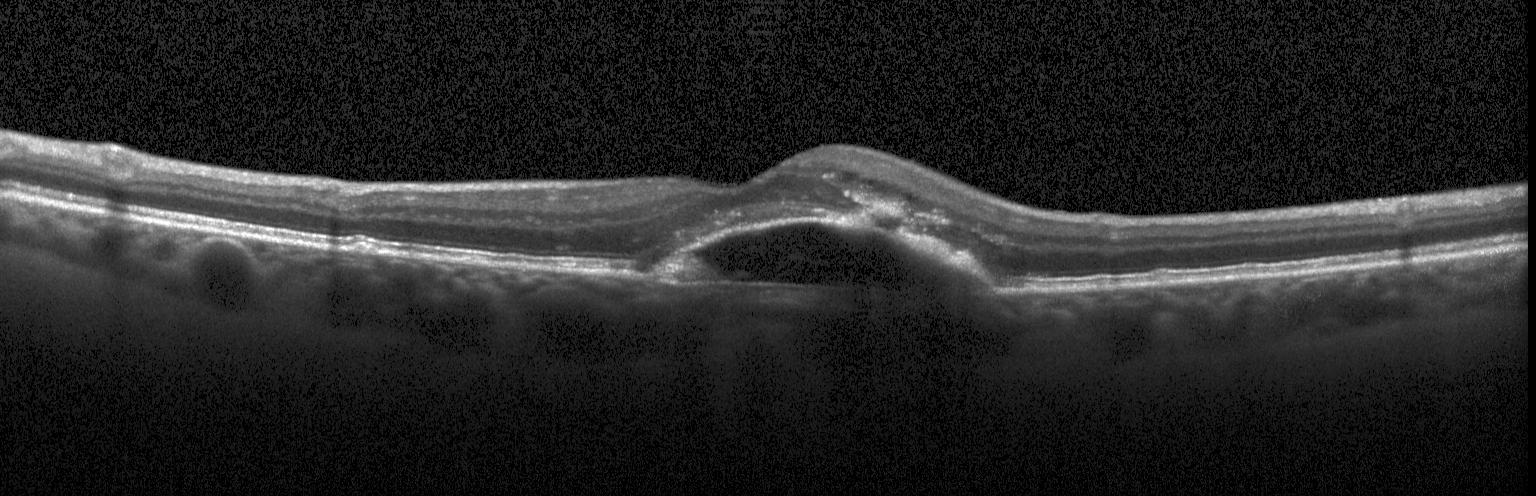 Horizontal scan through the fovea; optical coherence tomography B-scan; Heidelberg Spectralis
Diagnosis: a choroidal neovascular membrane.